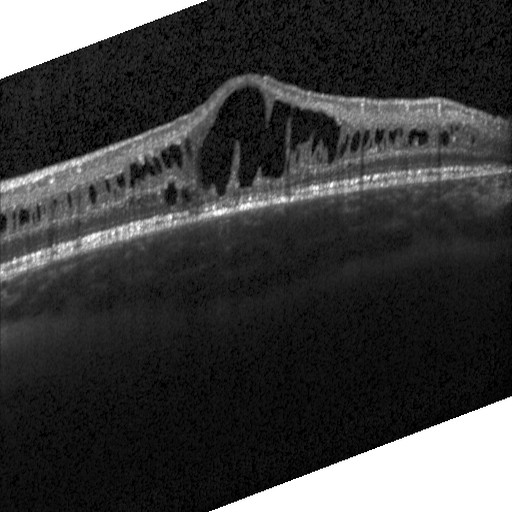
Retinal OCT B-scan. Impression: diabetic macular edema.